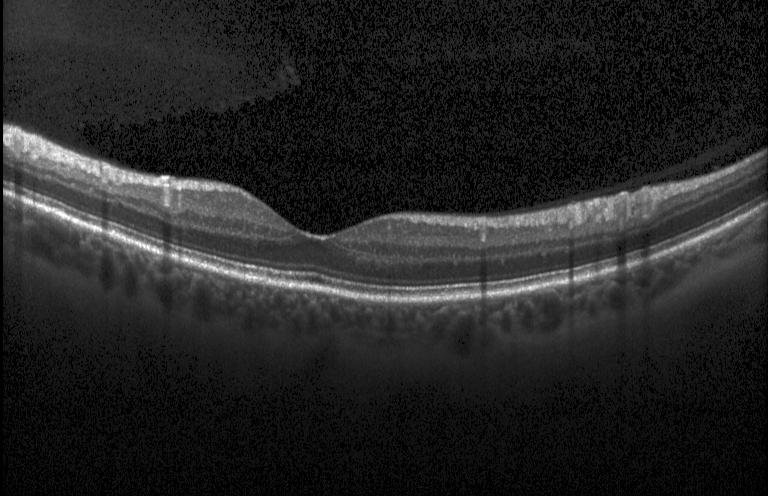
Retinal OCT cross-section
Macular OCT: neither choroidal neovascularization, diabetic macular edema, nor drusen.